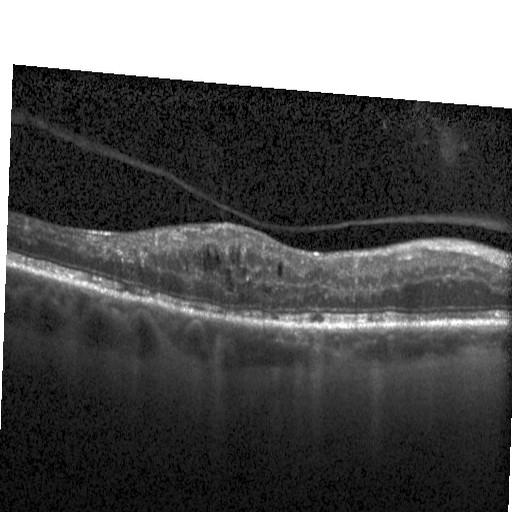

OCT line scan. Centered on the fovea
Diagnosis: diabetic macular edema.